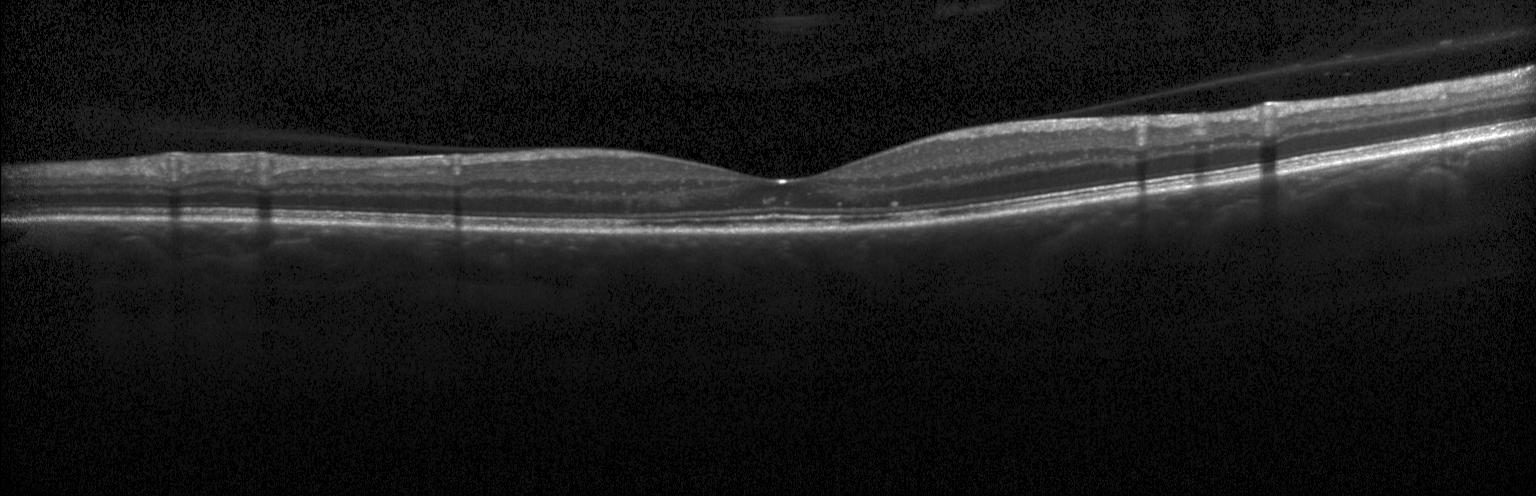 OCT B-scan, centered on the fovea, Heidelberg Spectralis.
The scan shows no evidence of choroidal neovascularization, diabetic macular edema, or drusen.